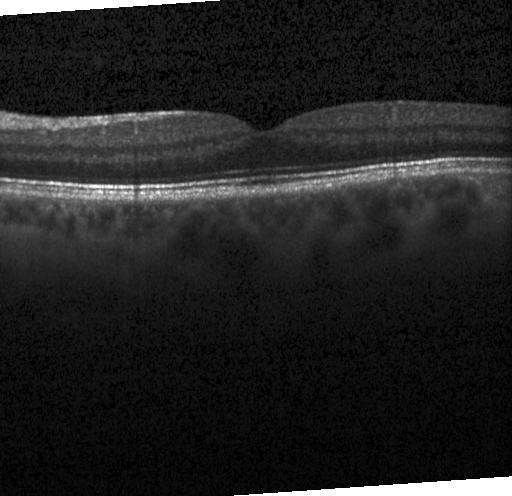
Heidelberg Spectralis, horizontal scan through the fovea, OCT line scan — Impression: no evidence of choroidal neovascularization, diabetic macular edema, or drusen.